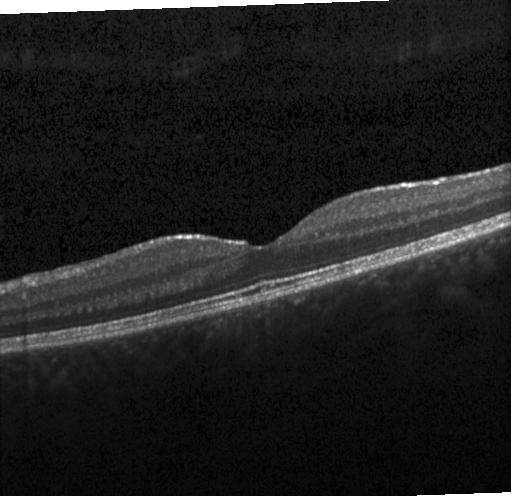
Through the macula, optical coherence tomography B-scan, Heidelberg Spectralis OCT system, spectral-domain optical coherence tomography — No evidence of choroidal neovascularization, diabetic macular edema, or drusen.